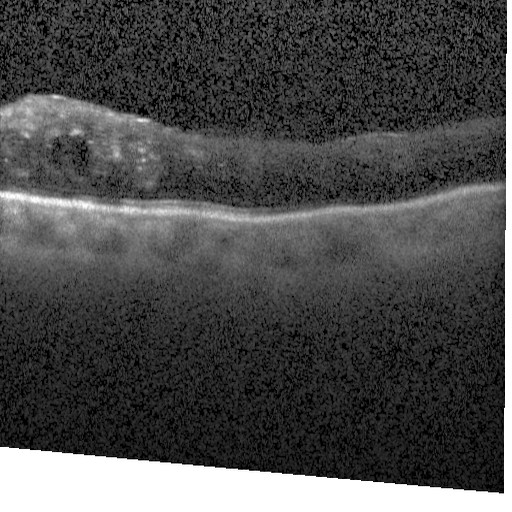 Dx: diabetic macular edema (DME).